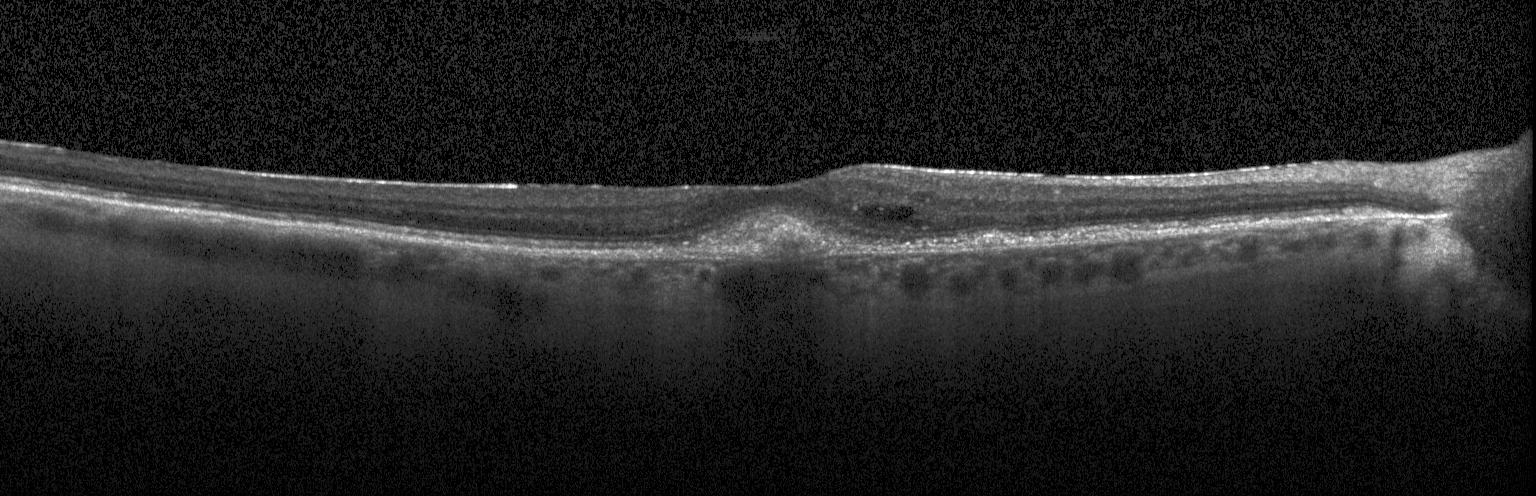
The scan shows choroidal neovascularization (CNV).